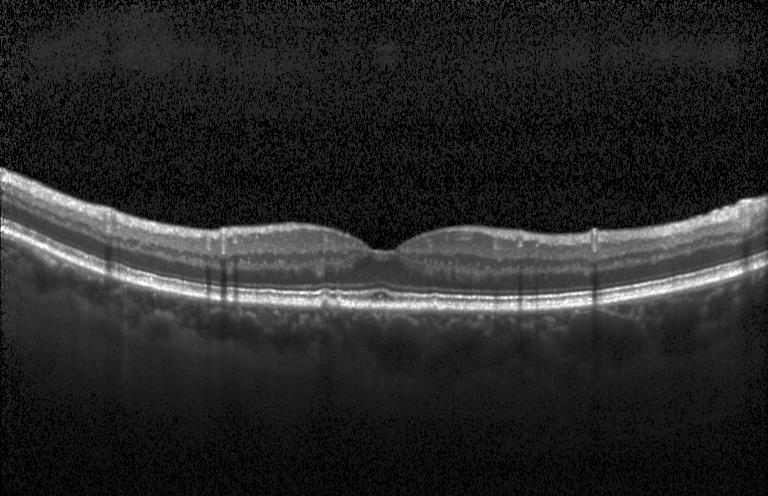

Heidelberg Spectralis · OCT line scan · spectral-domain optical coherence tomography — This B-scan demonstrates multiple drusen.